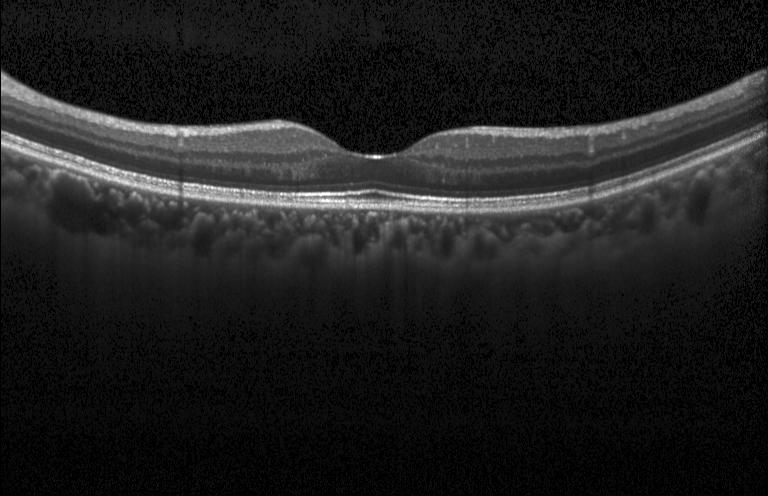 Diagnosis: no CNV, DME, or drusen.